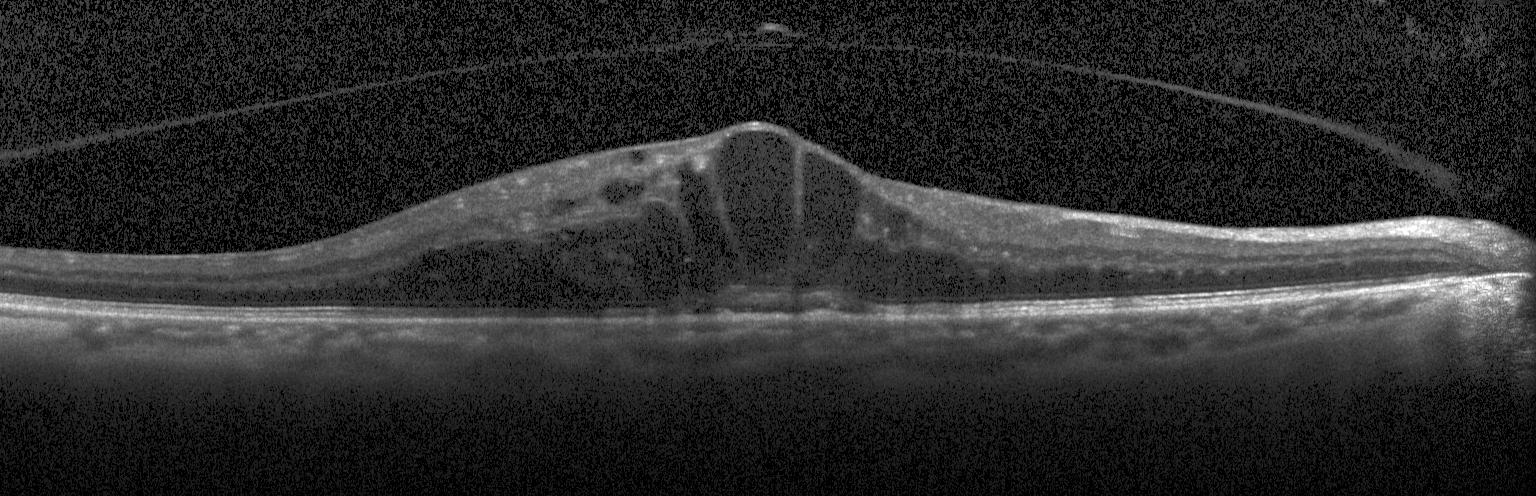
Diagnosis: diabetic macular edema.